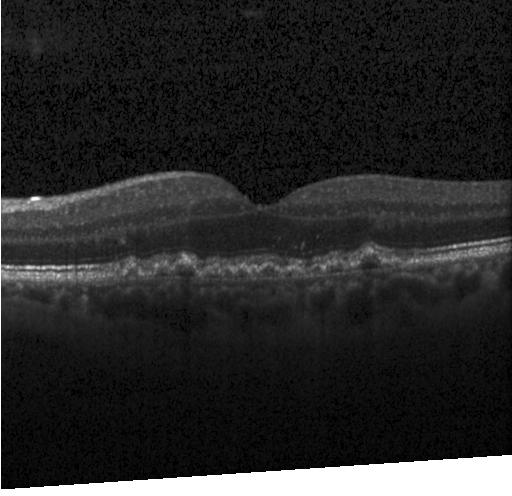

Impression: sub-RPE drusenoid deposits.